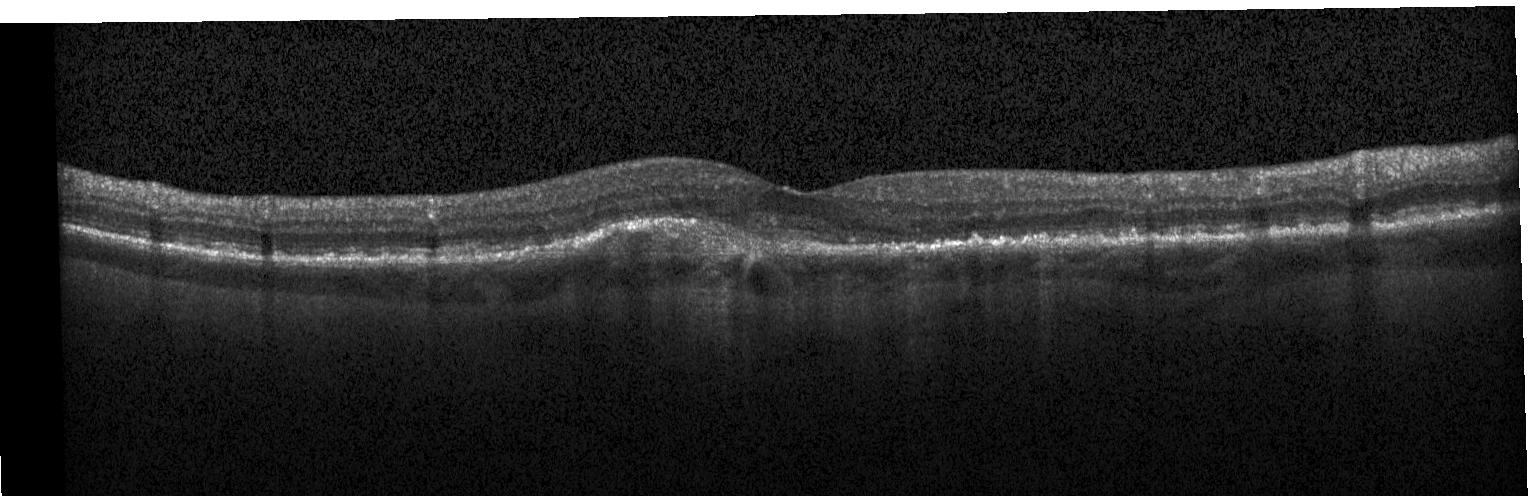

Impression: a choroidal neovascular membrane.